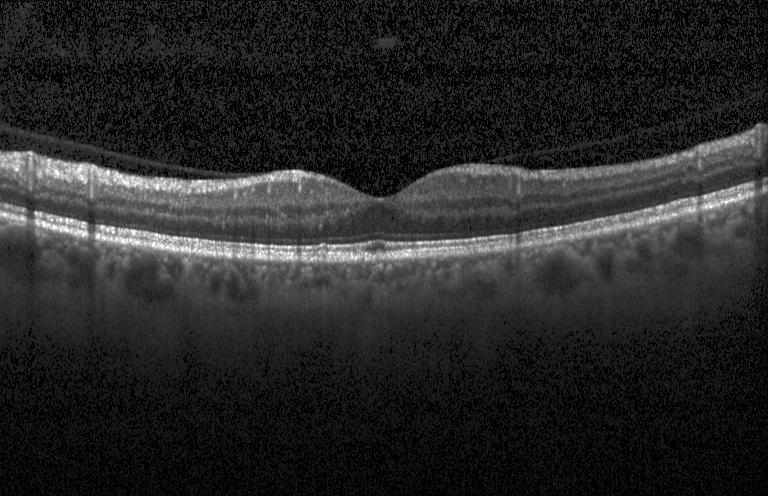
Spectral-domain OCT B-scan: neither choroidal neovascularization, diabetic macular edema, nor drusen.